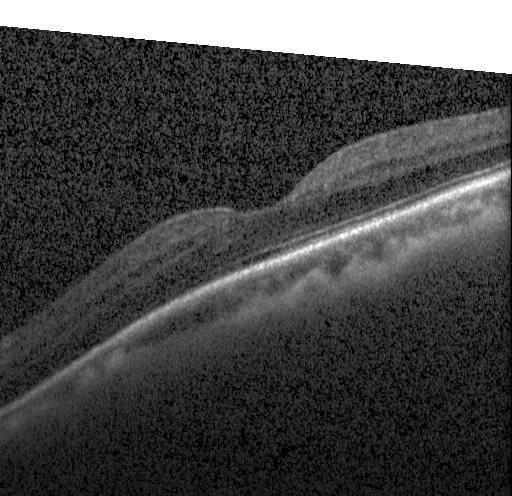
Optical coherence tomography scan
No choroidal neovascularization, diabetic macular edema, or drusen.